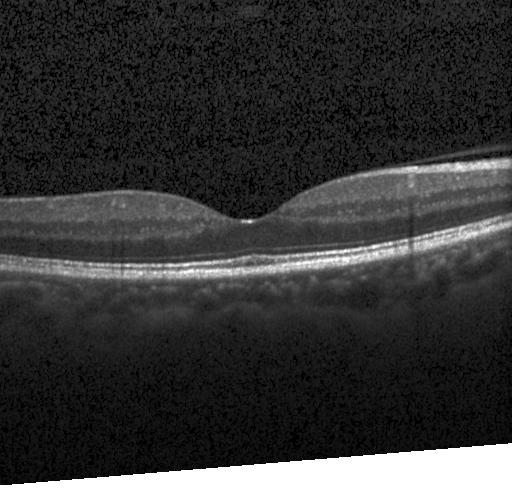
Impression: no choroidal neovascularization, no diabetic macular edema, and no drusen.